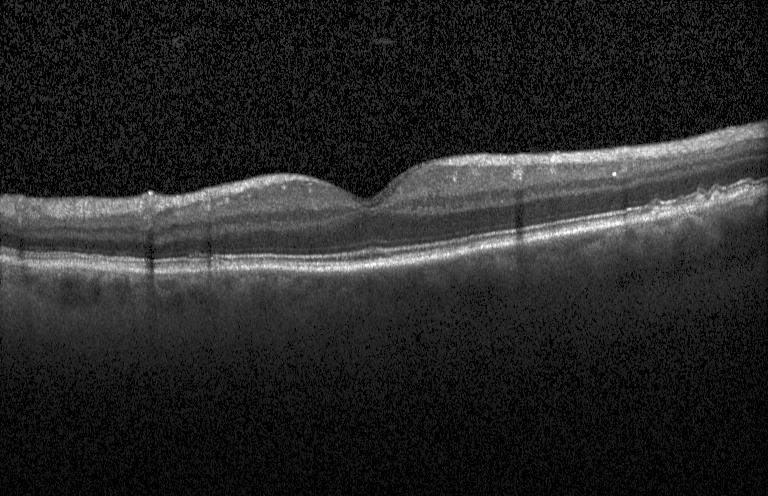
Impression: sub-RPE drusenoid deposits.